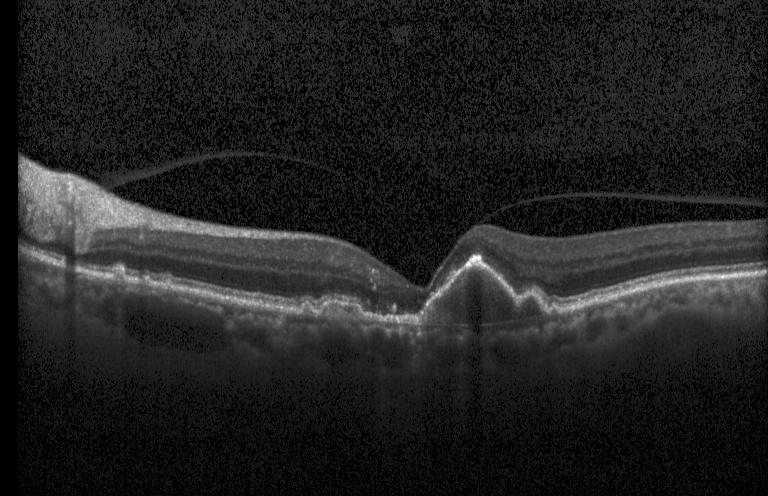 OCT B-scan — Diagnosis: CNV.